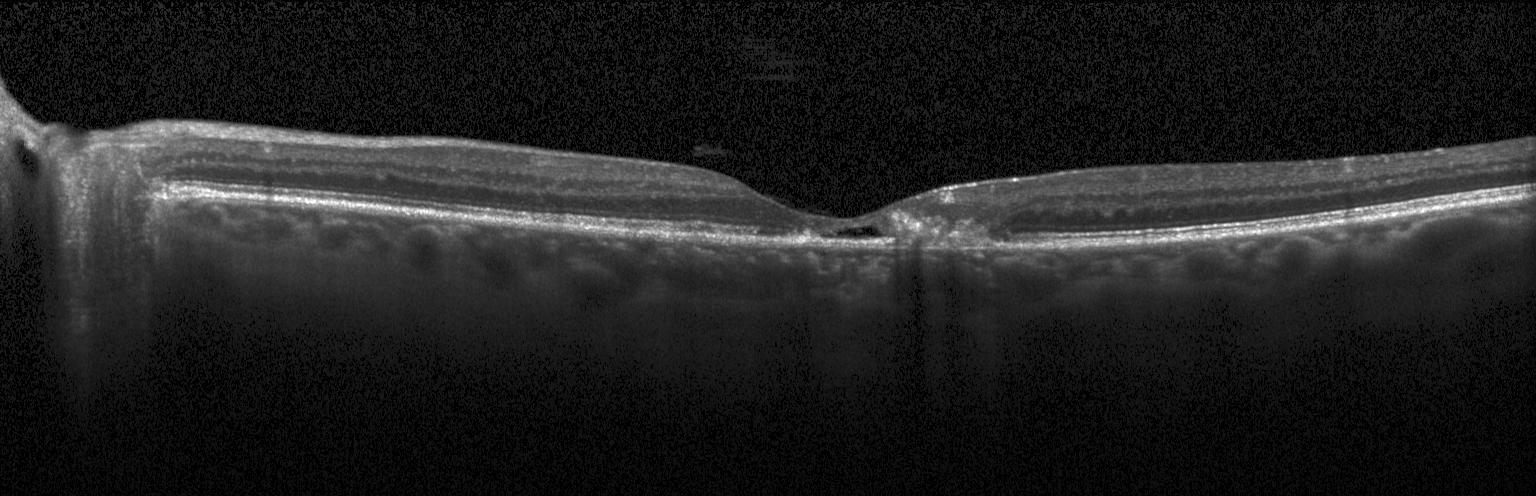 Centered on the fovea, Heidelberg Spectralis, SD-OCT, OCT B-scan
Macular OCT: a choroidal neovascular membrane.